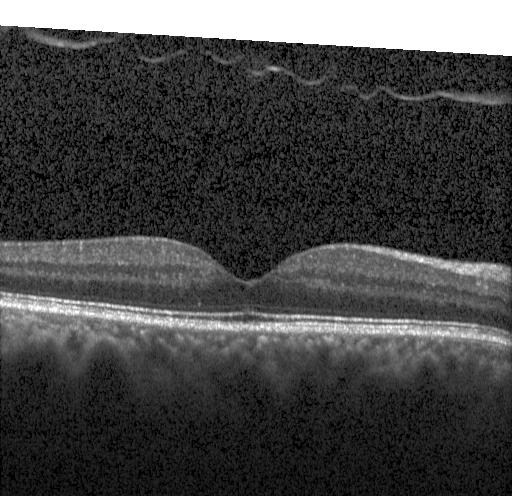
Horizontal scan through the fovea. Heidelberg Spectralis OCT system. OCT line scan. Spectral-domain OCT. The scan shows no evidence of choroidal neovascularization, diabetic macular edema, or drusen.